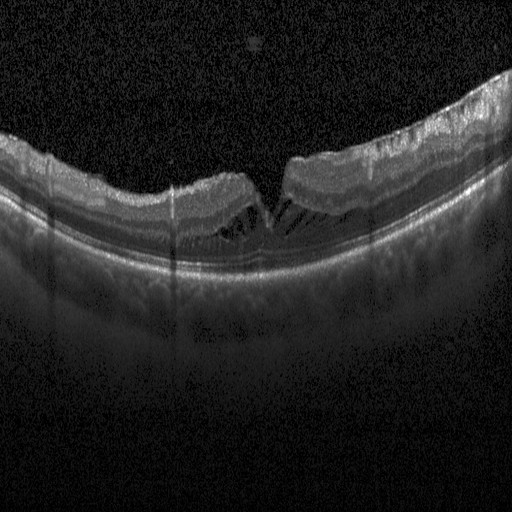 Diagnosis: DME.